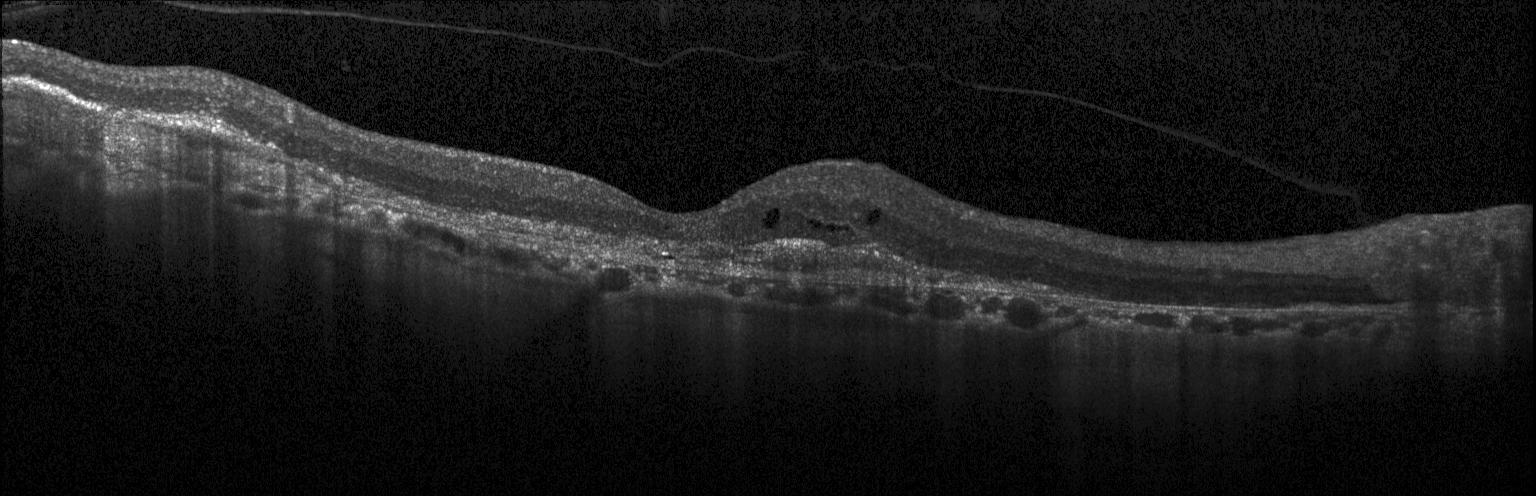

Macular scan; optical coherence tomography B-scan.
The scan shows CNV.